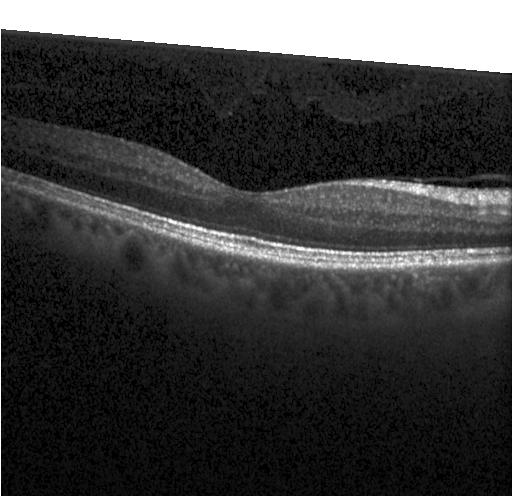

Diagnosis: no choroidal neovascularization, diabetic macular edema, or drusen.